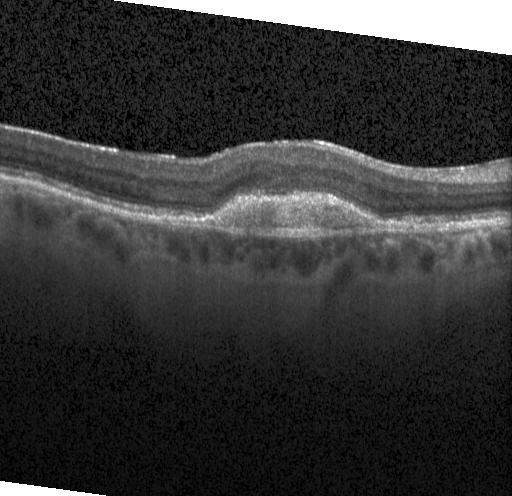
OCT line scan, acquired on a Heidelberg Spectralis.
Finding: a choroidal neovascular membrane.